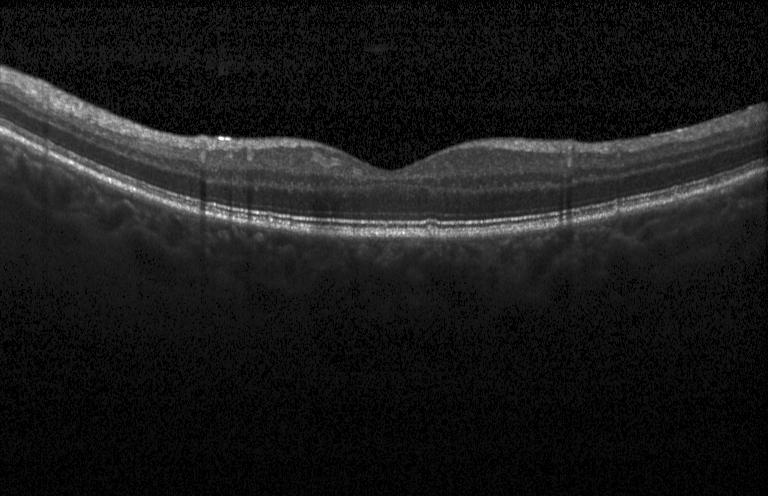 Optical coherence tomography B-scan
OCT finding: no choroidal neovascularization, diabetic macular edema, or drusen.